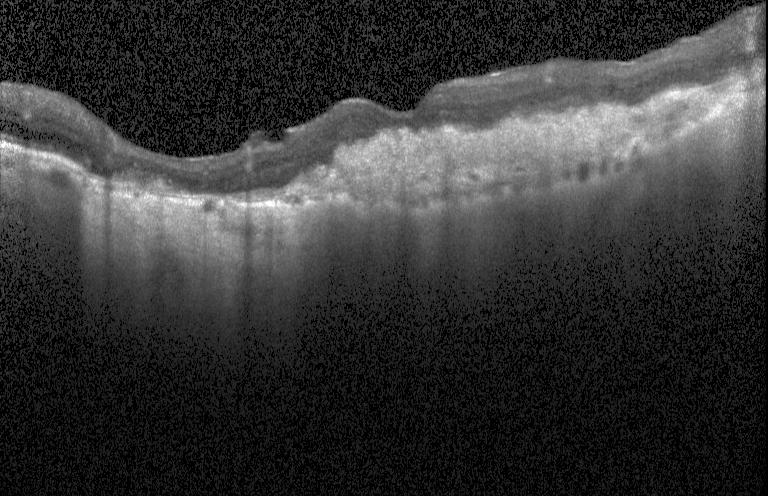
Retinal OCT B-scan, SD-OCT, macular scan. Diagnosis: CNV.